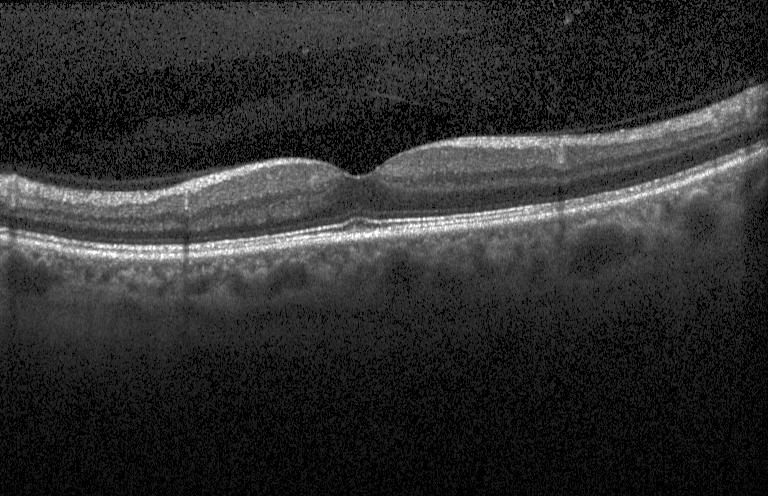

Spectral-domain optical coherence tomography, acquired on a Heidelberg Spectralis, optical coherence tomography scan, fovea-centered. No choroidal neovascularization, diabetic macular edema, or drusen.